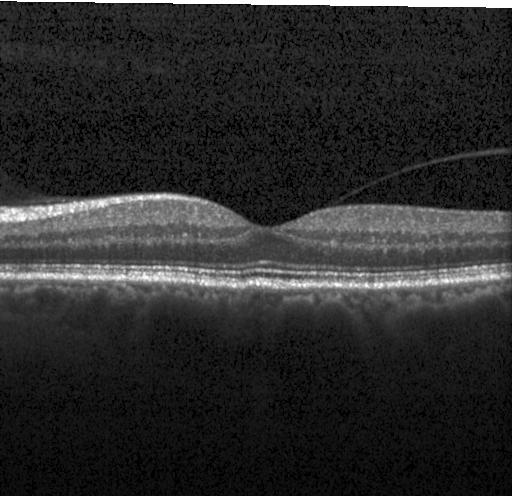

OCT finding: no evidence of choroidal neovascularization, diabetic macular edema, or drusen.